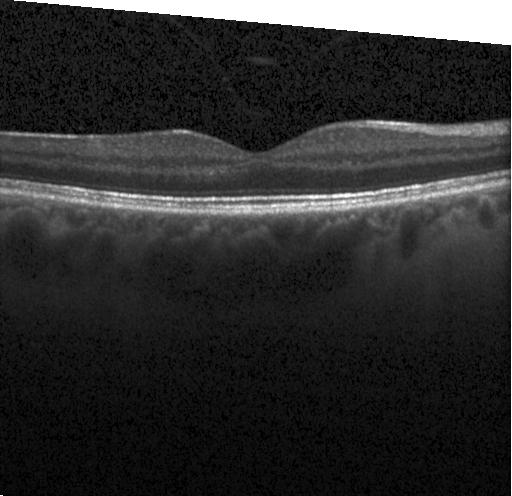

Spectral-domain OCT B-scan: no evidence of CNV, DME, or drusen.